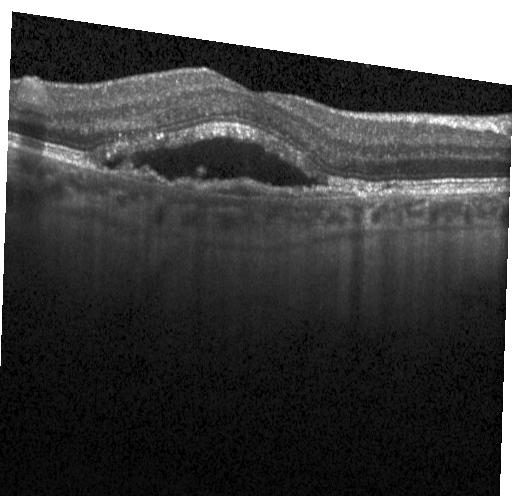 Spectral-domain OCT. Optical coherence tomography scan
Macular OCT: a choroidal neovascular membrane.